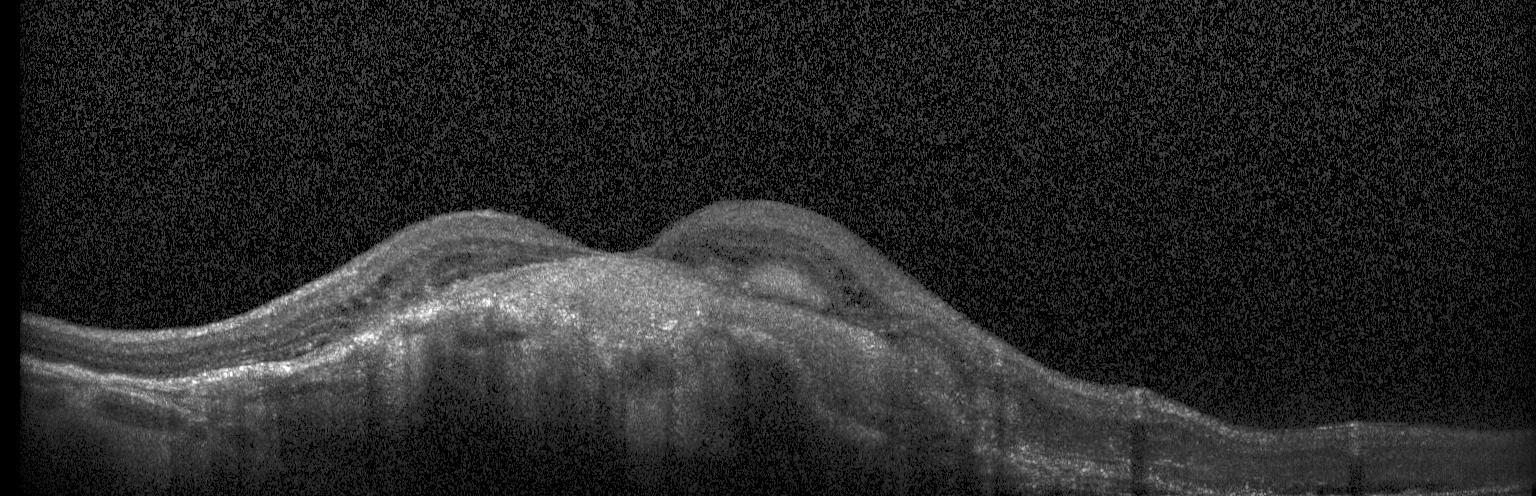 Through the macula; Heidelberg Spectralis OCT system; retinal OCT cross-section
Dx: choroidal neovascularization (CNV).